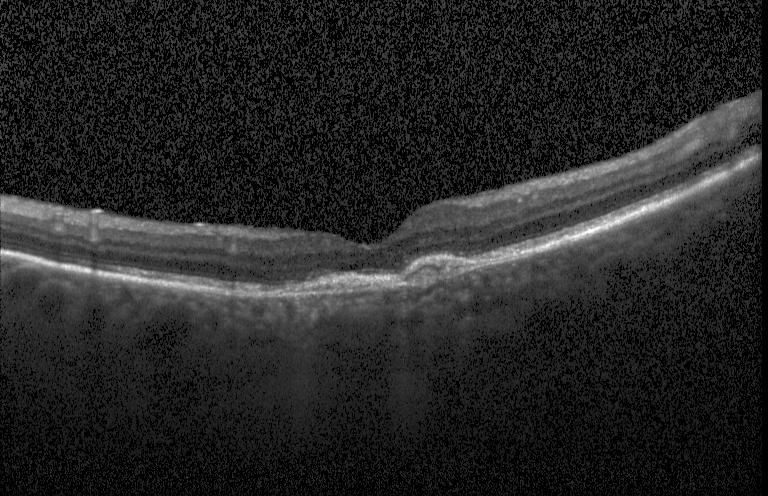

Heidelberg Spectralis OCT system. Optical coherence tomography B-scan. Spectral-domain OCT. Macular scan
Macular OCT: a choroidal neovascular membrane.